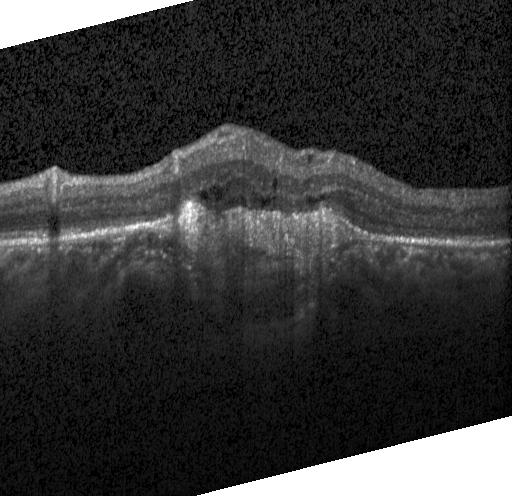 A choroidal neovascular membrane.